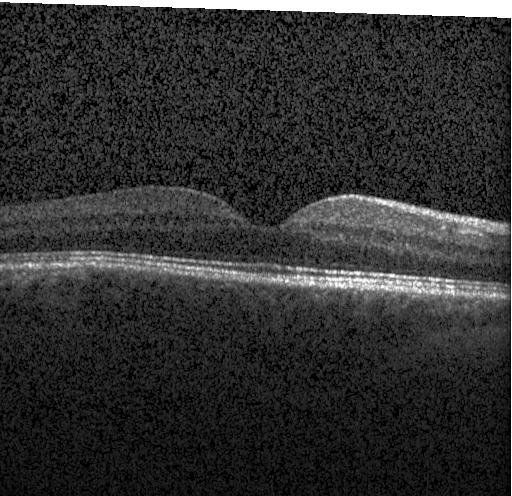

No evidence of choroidal neovascularization, diabetic macular edema, or drusen.